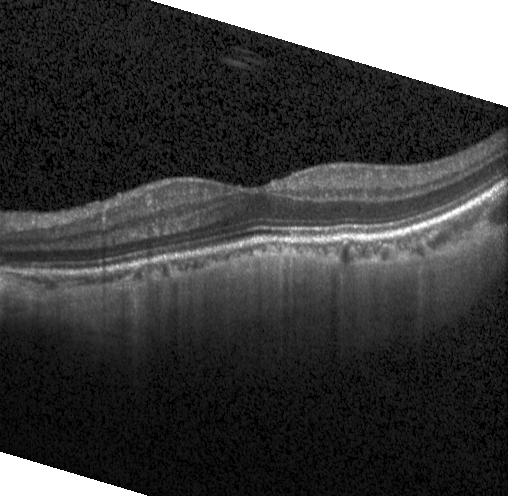
Spectral-domain OCT, through the macula, optical coherence tomography scan, acquired on a Heidelberg Spectralis
Neither choroidal neovascularization, diabetic macular edema, nor drusen.